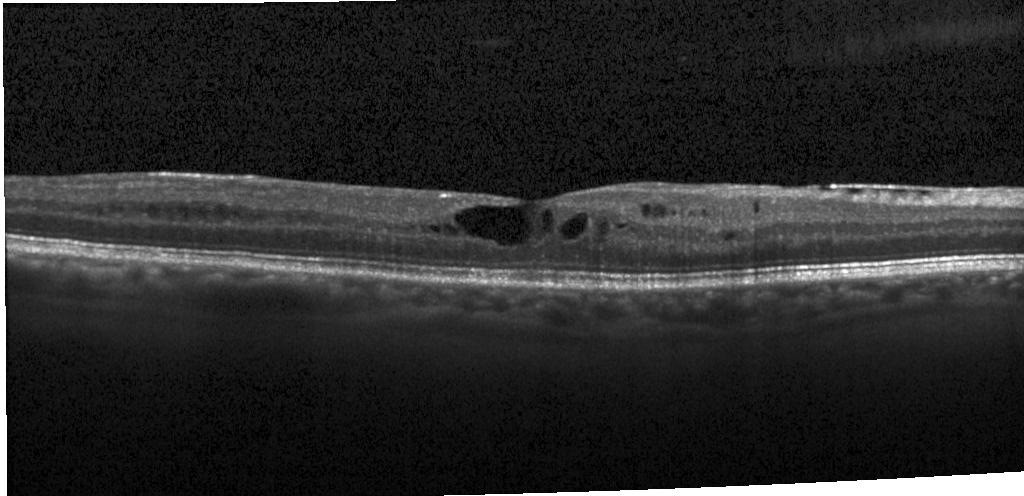 Through the macula, Heidelberg Spectralis OCT system, spectral-domain optical coherence tomography, retinal OCT B-scan — Assessment: diabetic macular edema.